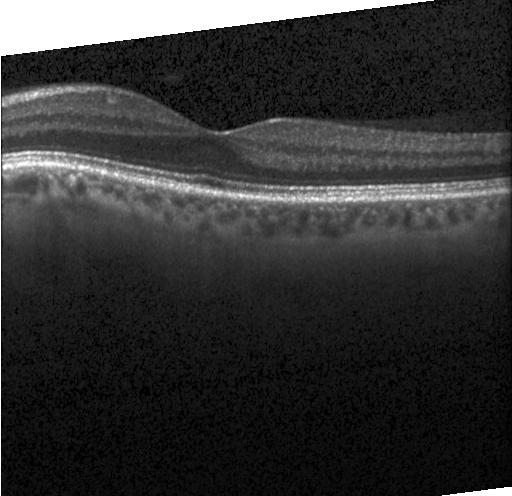

OCT B-scan. Fovea-centered. Spectral-domain optical coherence tomography. Instrument: Heidelberg Spectralis
Diagnosis: no choroidal neovascularization, no diabetic macular edema, and no drusen.